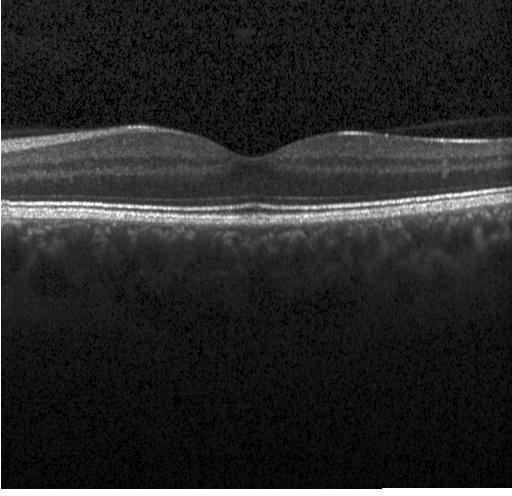 OCT finding: no evidence of CNV, DME, or drusen.